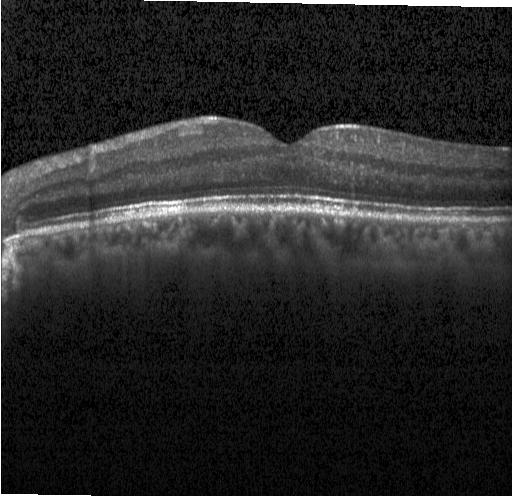

Impression: no choroidal neovascularization, diabetic macular edema, or drusen.